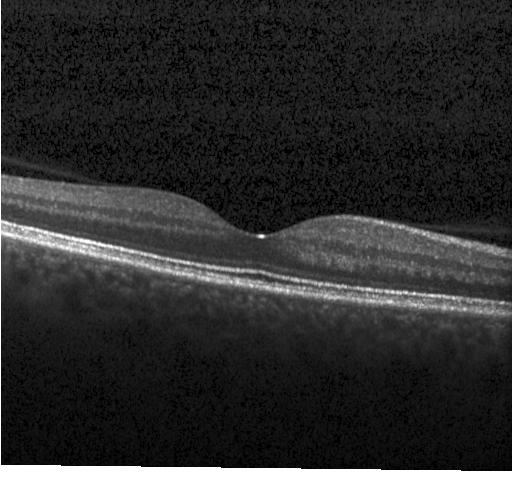
Heidelberg Spectralis. OCT line scan. Through the macula.
Assessment: no choroidal neovascularization, diabetic macular edema, or drusen.